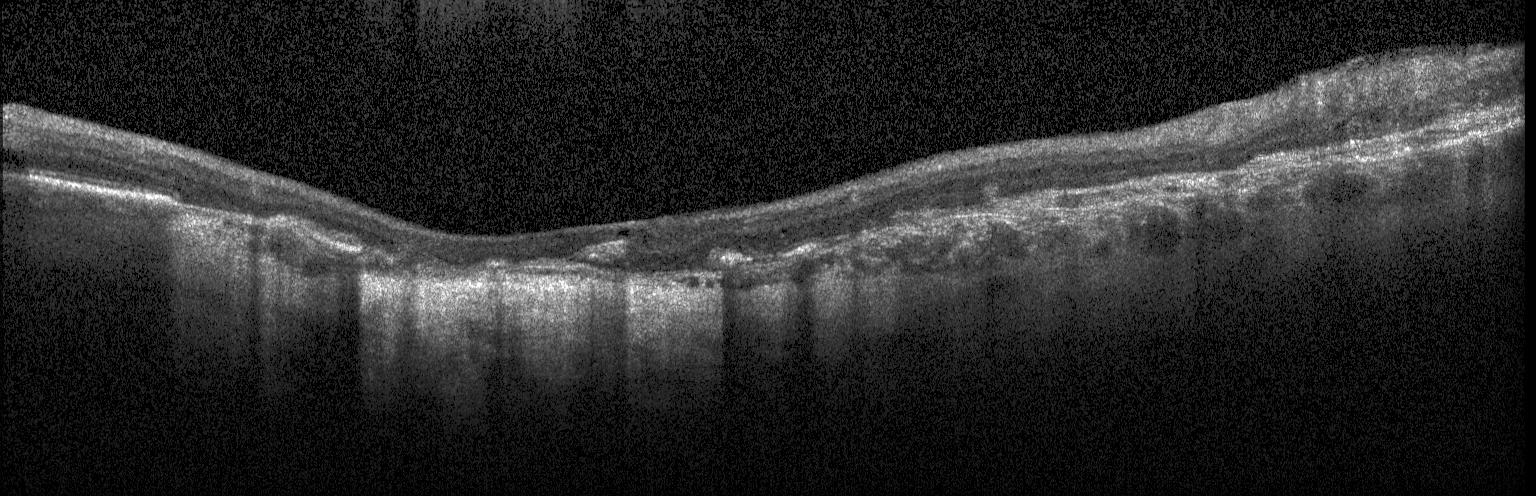 Diagnosis: choroidal neovascularization.